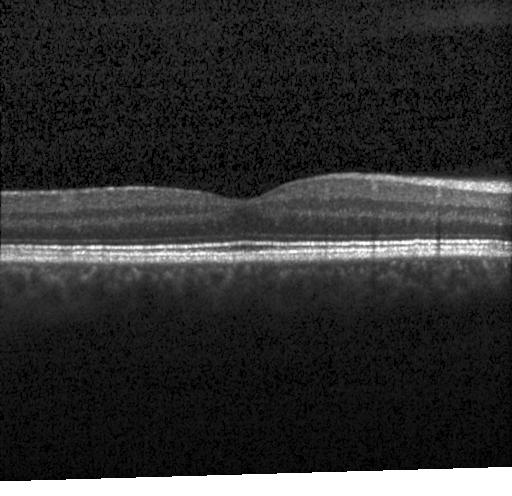
Retinal OCT cross-section — OCT finding: no choroidal neovascularization, no diabetic macular edema, and no drusen.